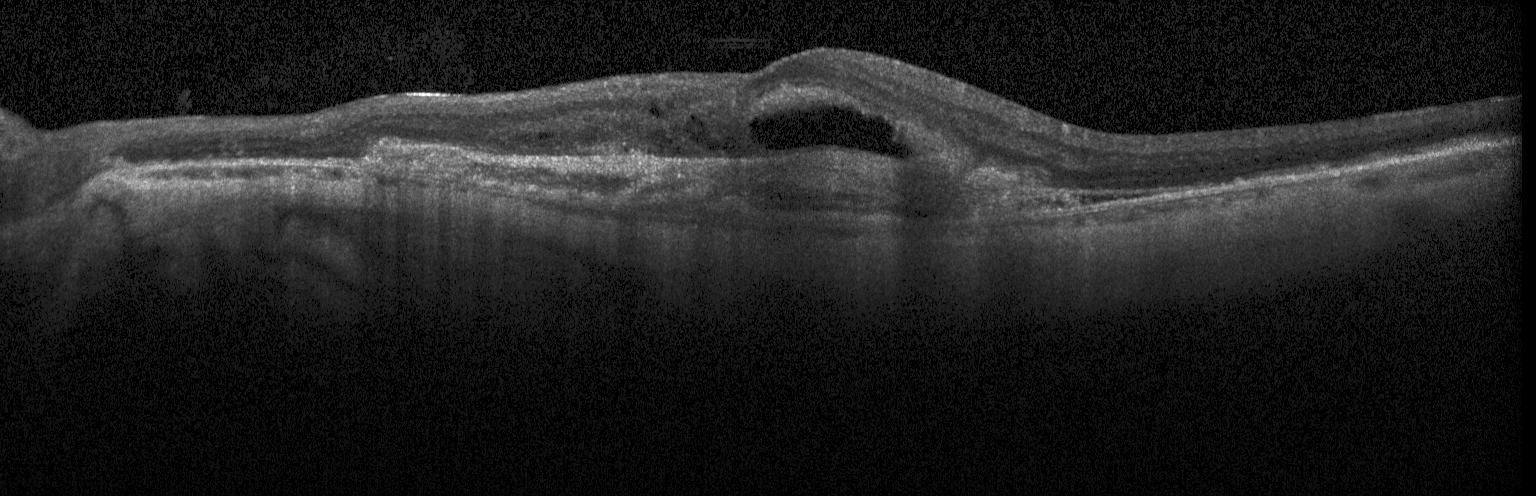 Optical coherence tomography B-scan, Heidelberg Spectralis OCT system, through the macula, spectral-domain optical coherence tomography — Dx: choroidal neovascularization (CNV).